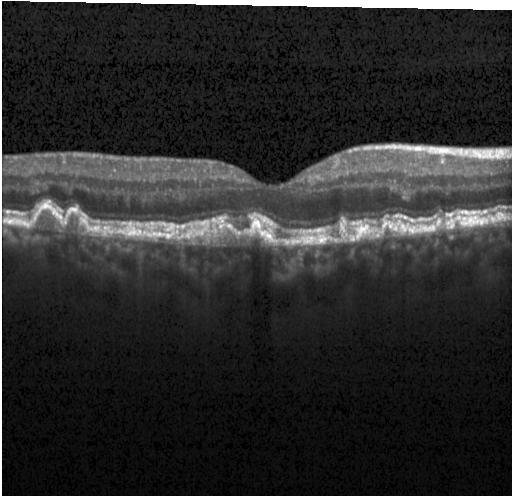
Impression: drusen.